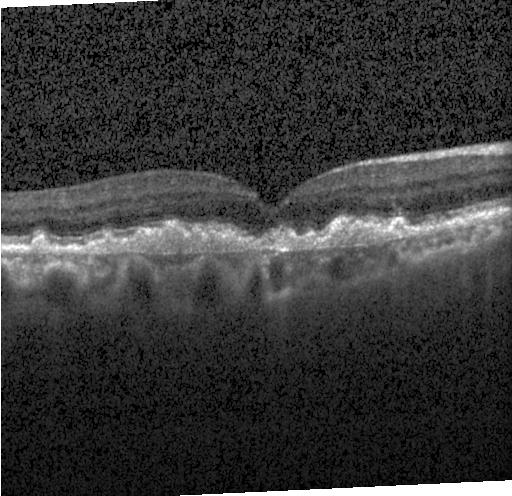

A choroidal neovascular membrane.